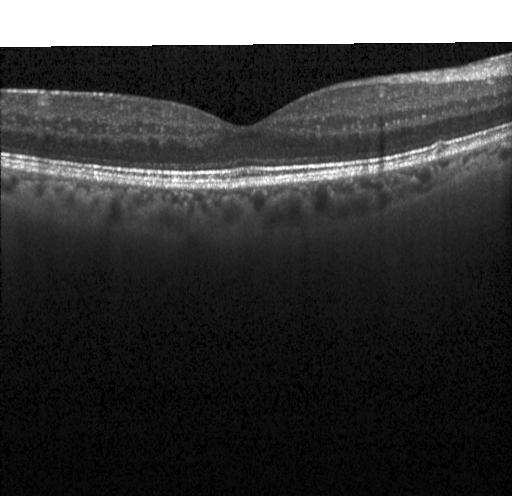 Retinal OCT cross-section. SD-OCT. Instrument: Heidelberg Spectralis. Centered on the fovea.
Diagnosis: no choroidal neovascularization, no diabetic macular edema, and no drusen.